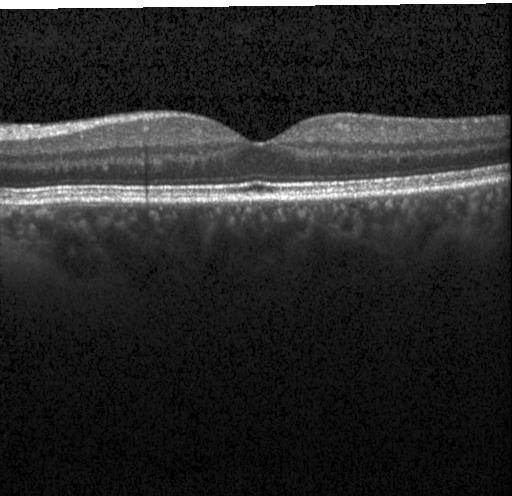
Diagnosis: no choroidal neovascularization, no diabetic macular edema, and no drusen.